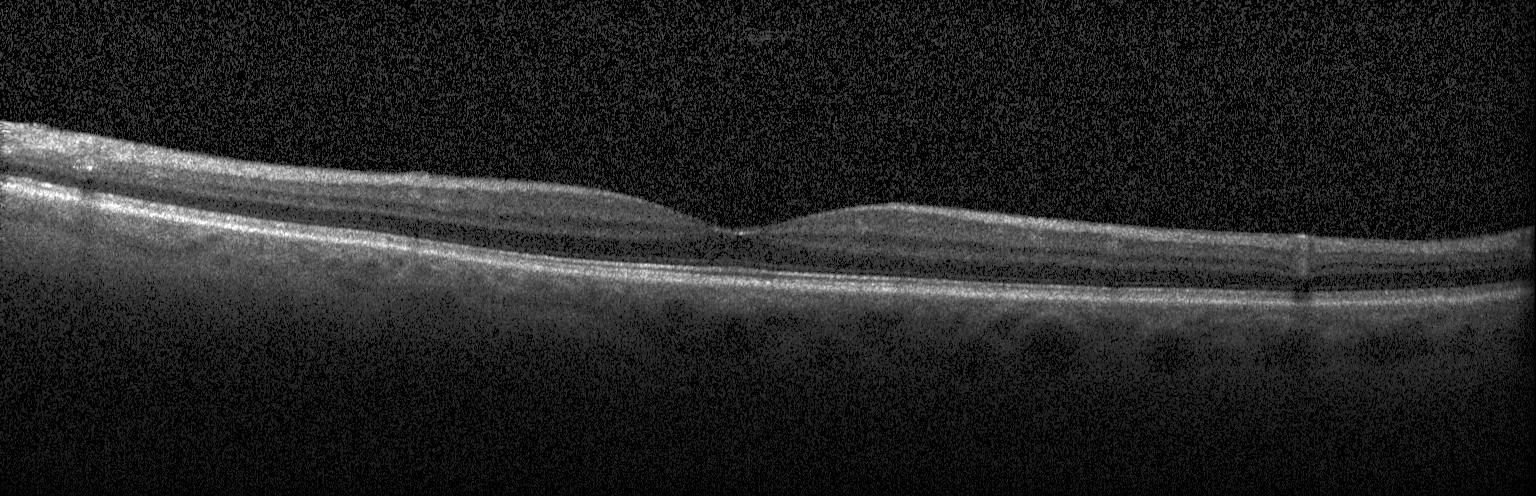
Impression: no choroidal neovascularization, diabetic macular edema, or drusen.